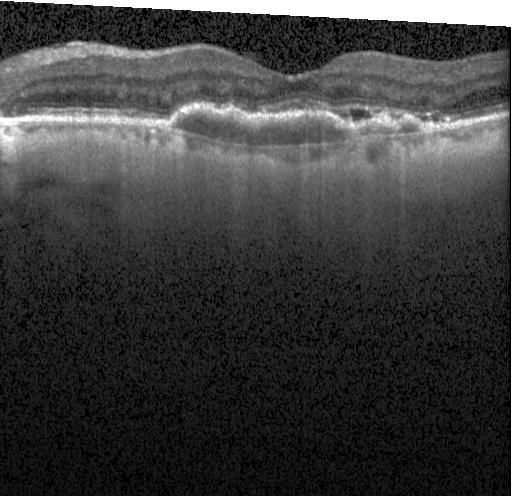
Retinal OCT B-scan; horizontal scan through the fovea; spectral-domain optical coherence tomography; Heidelberg Spectralis OCT system
This B-scan demonstrates CNV.